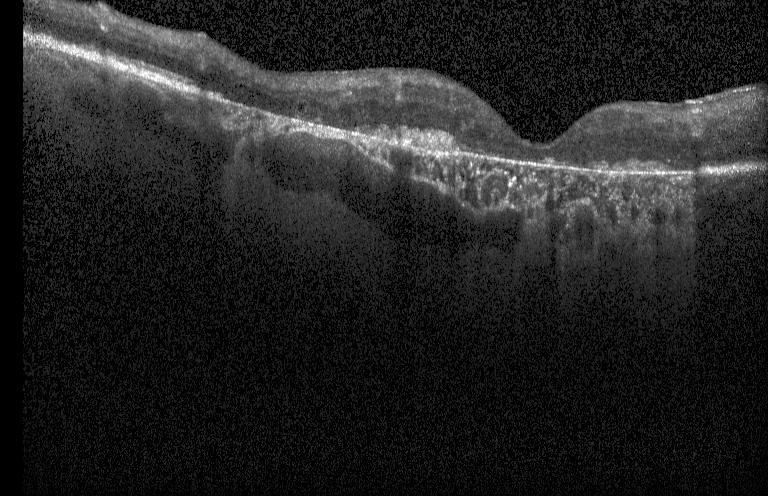
A choroidal neovascular membrane.